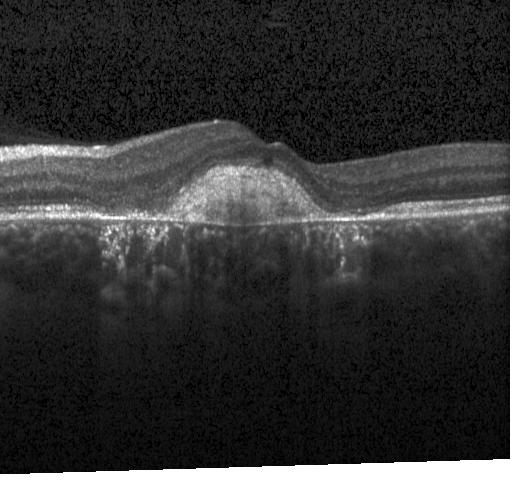 Macular scan, SD-OCT, OCT B-scan — Diagnosis: choroidal neovascularization (CNV).